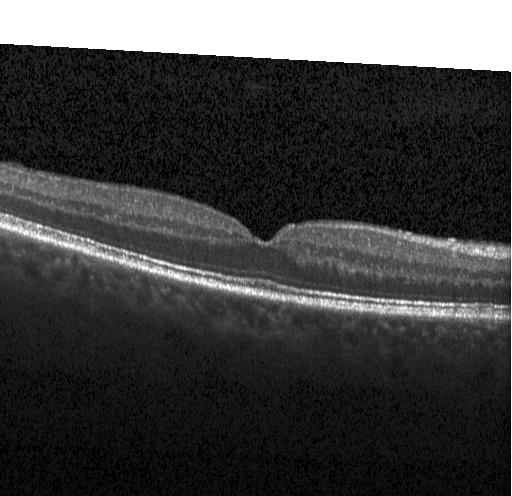 OCT scan showing no choroidal neovascularization, no diabetic macular edema, and no drusen.